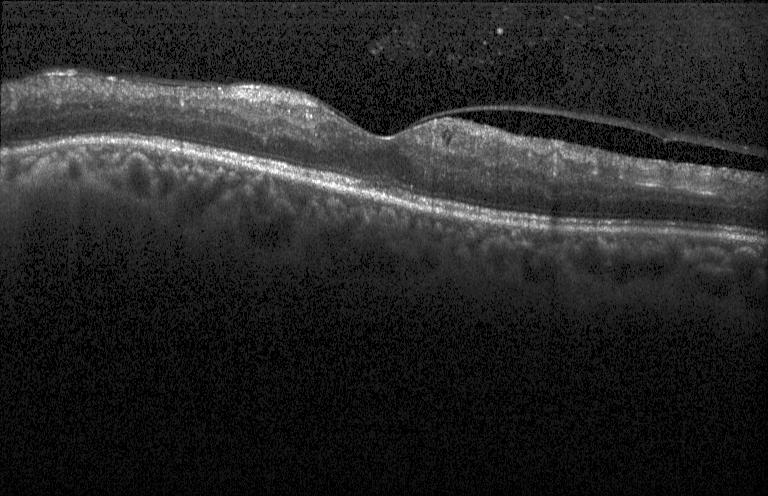
Spectral-domain OCT B-scan: diabetic macular edema.